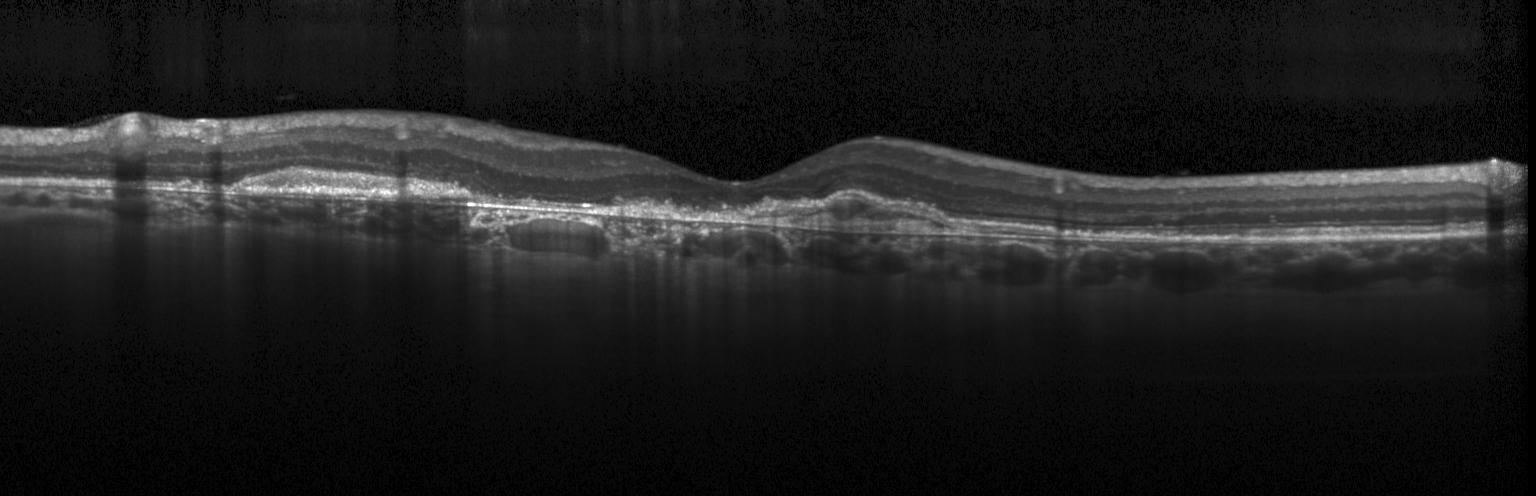
Spectral-domain OCT, OCT B-scan. Assessment: a choroidal neovascular membrane.